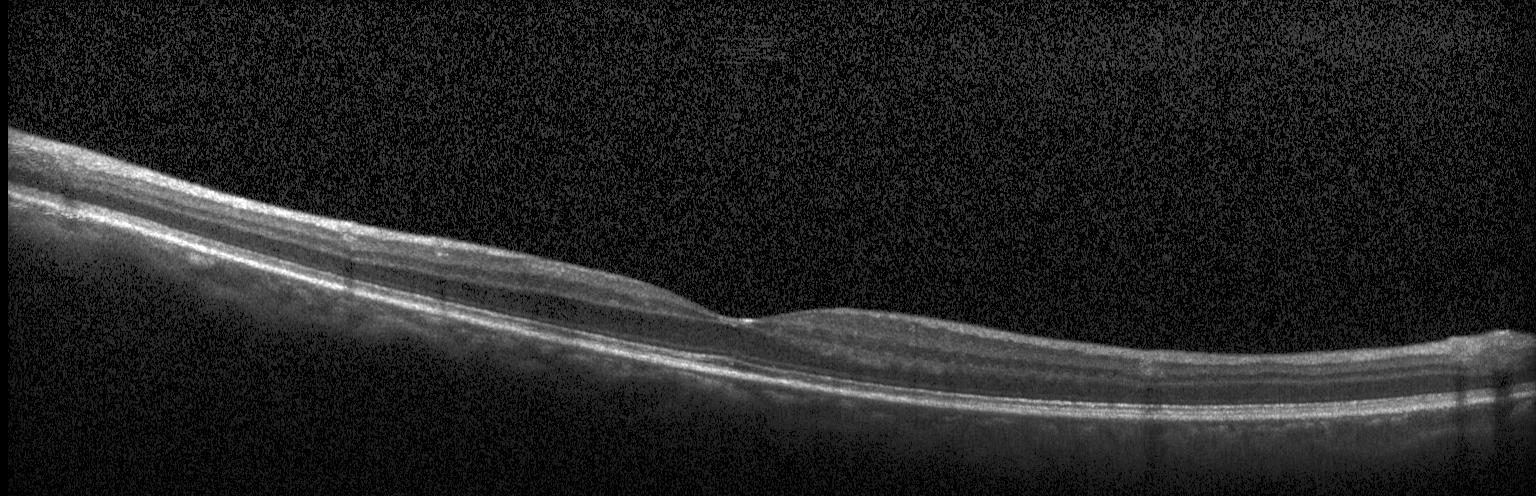
SD-OCT · retinal OCT cross-section · macular scan · Heidelberg Spectralis OCT system.
Diagnosis: no choroidal neovascularization, no diabetic macular edema, and no drusen.